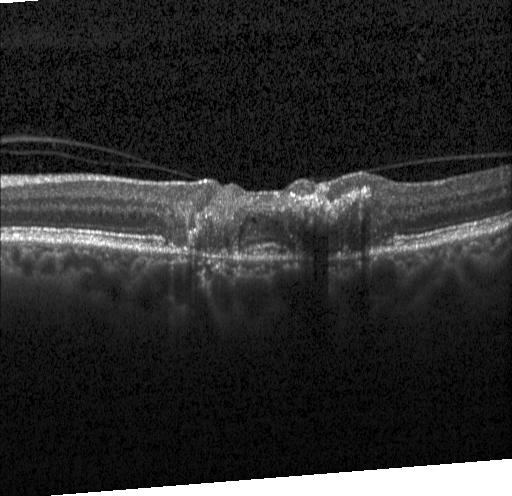
Optical coherence tomography scan — Impression: a choroidal neovascular membrane.